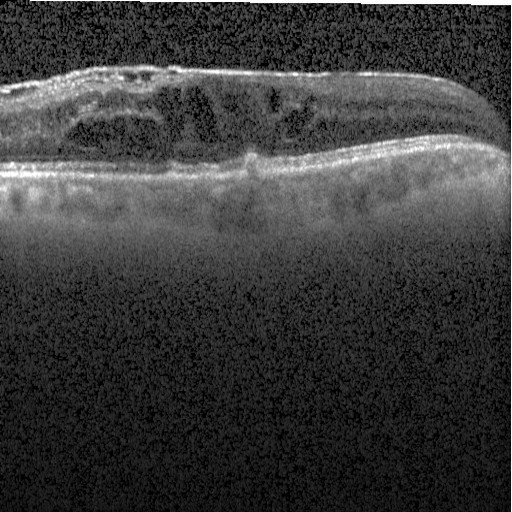 Diagnosis: diabetic macular edema.